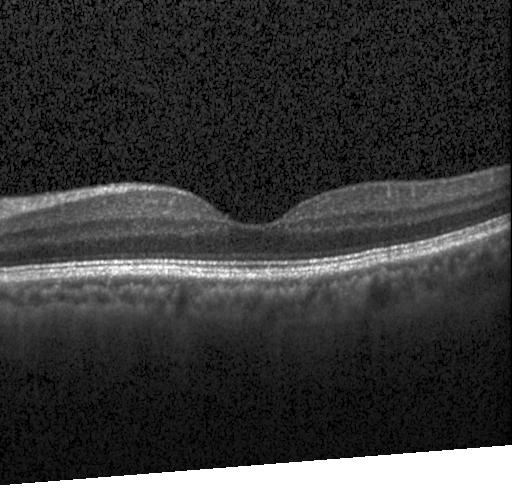

Fovea-centered, spectral-domain optical coherence tomography, retinal OCT B-scan, instrument: Heidelberg Spectralis
Finding: neither CNV, DME, nor drusen.